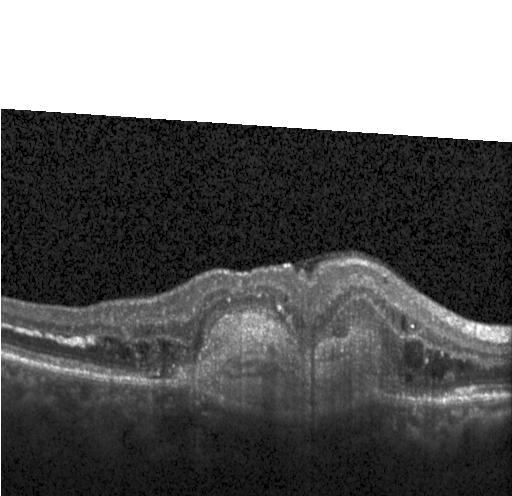
Diagnosis: CNV.